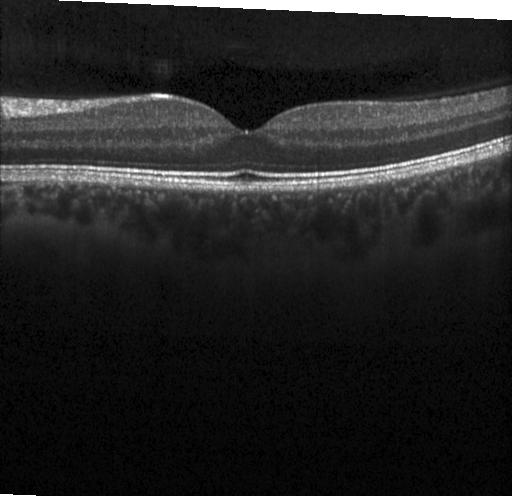 Spectral-domain OCT B-scan: no choroidal neovascularization, no diabetic macular edema, and no drusen.